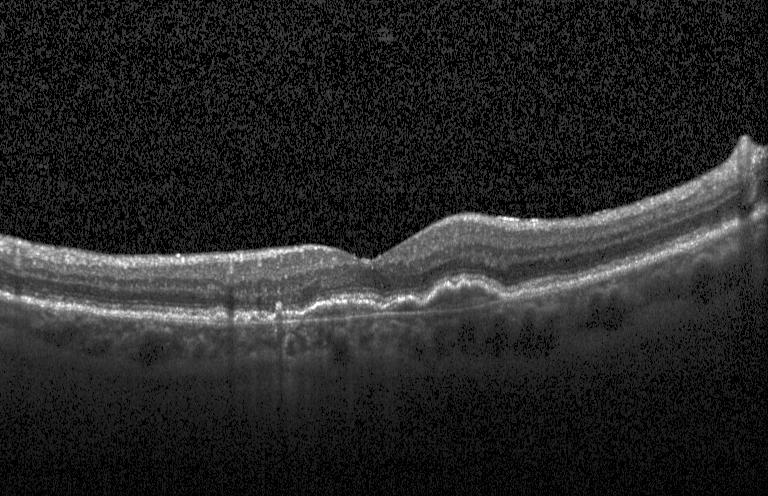 Finding: choroidal neovascularization (CNV).